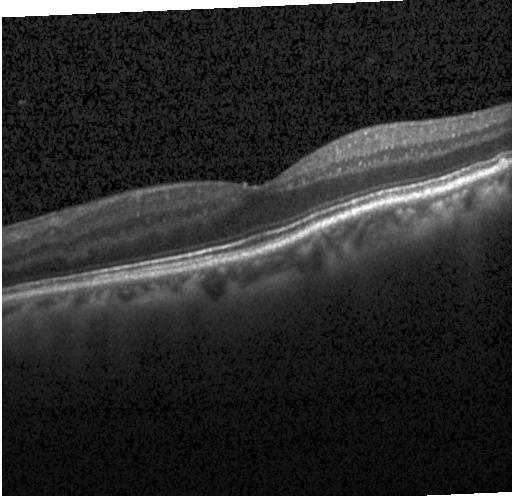

Macular OCT demonstrating neither choroidal neovascularization, diabetic macular edema, nor drusen.